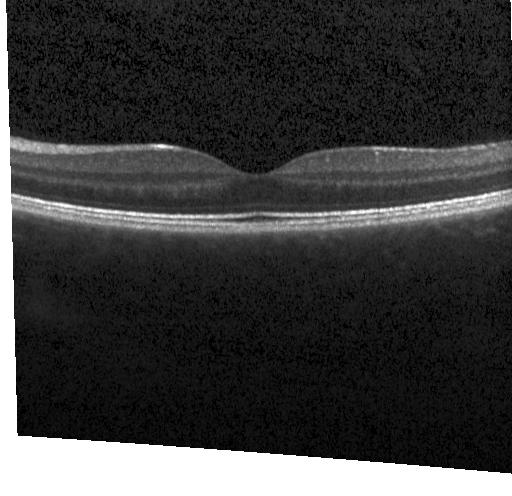 Optical coherence tomography B-scan; through the macula; Heidelberg Spectralis OCT system; spectral-domain OCT — Finding: no evidence of choroidal neovascularization, diabetic macular edema, or drusen.